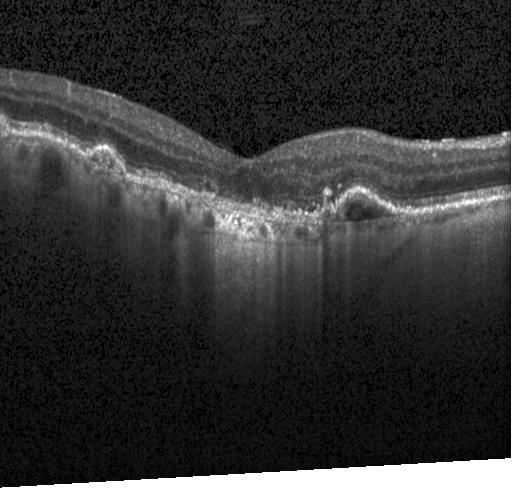 Retinal OCT B-scan, horizontal scan through the fovea, spectral-domain OCT — The scan shows a choroidal neovascular membrane.